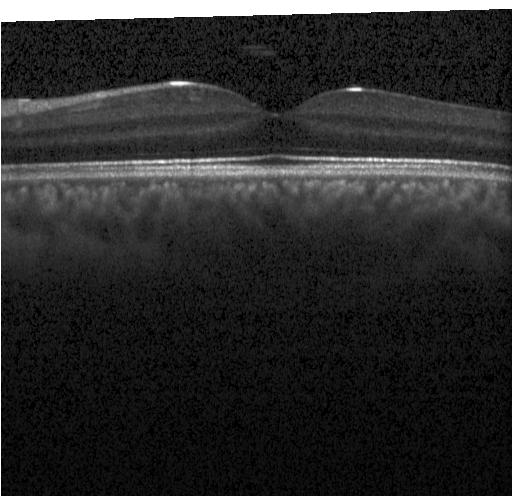 OCT finding: no choroidal neovascularization, no diabetic macular edema, and no drusen.